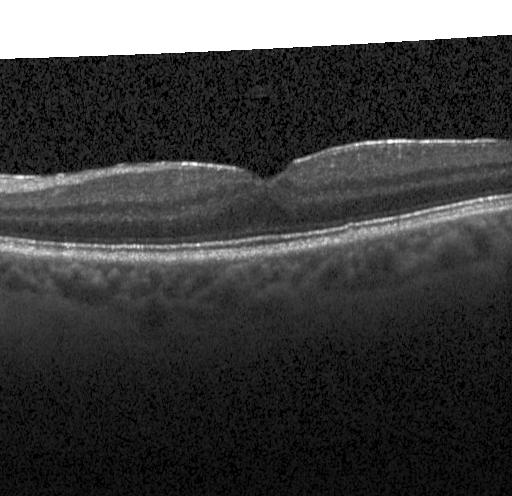 Optical coherence tomography B-scan. Heidelberg Spectralis
Diagnosis: no choroidal neovascularization, no diabetic macular edema, and no drusen.